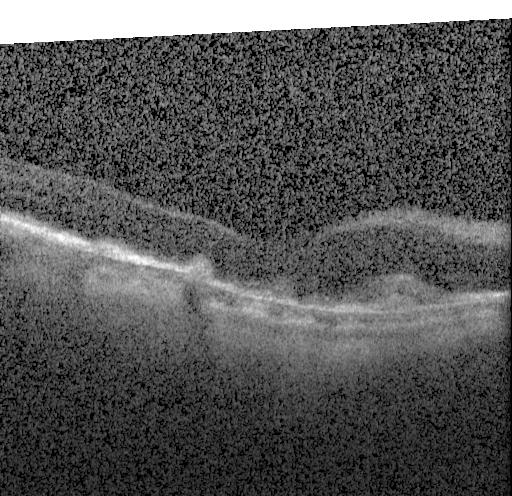 Retinal OCT cross-section · spectral-domain OCT — The scan shows choroidal neovascularization.